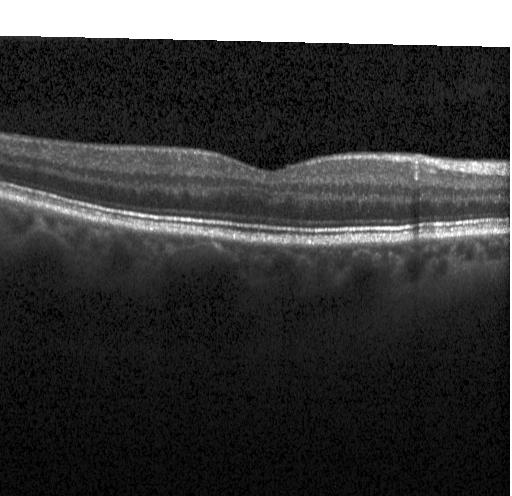

Fovea-centered · retinal OCT B-scan
Assessment: neither choroidal neovascularization, diabetic macular edema, nor drusen.